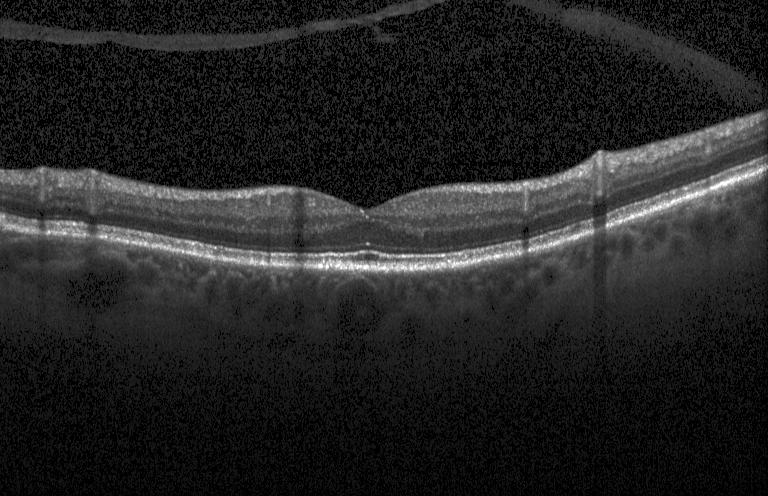
Macular OCT: neither CNV, DME, nor drusen.